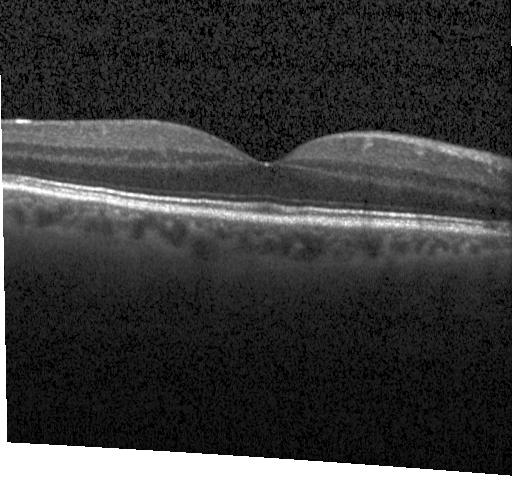

OCT B-scan
Macular OCT: no evidence of CNV, DME, or drusen.